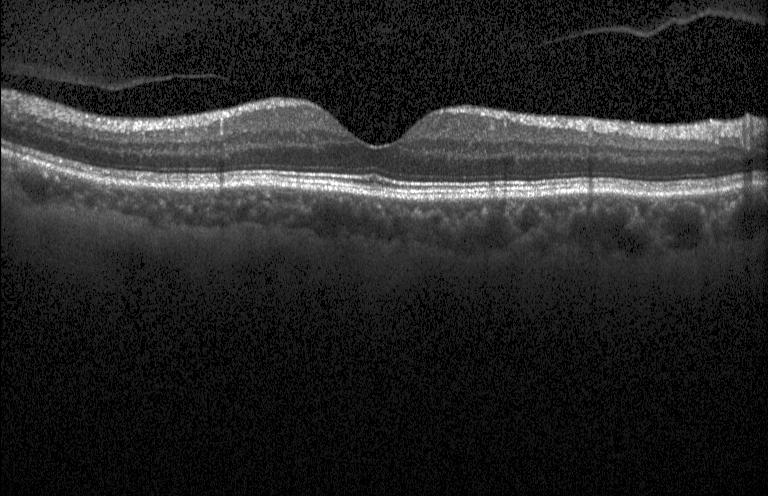

Diagnosis: no choroidal neovascularization, no diabetic macular edema, and no drusen.